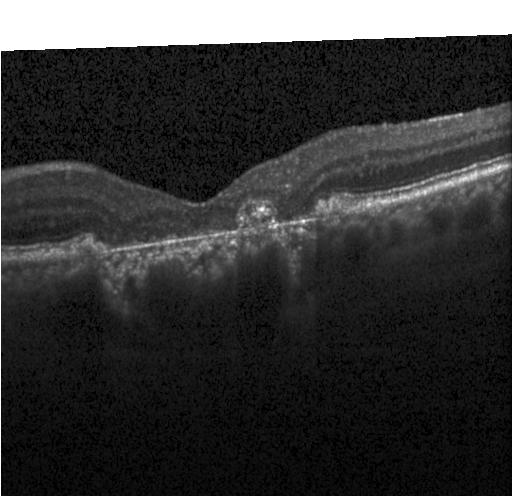

Macular OCT demonstrating CNV.